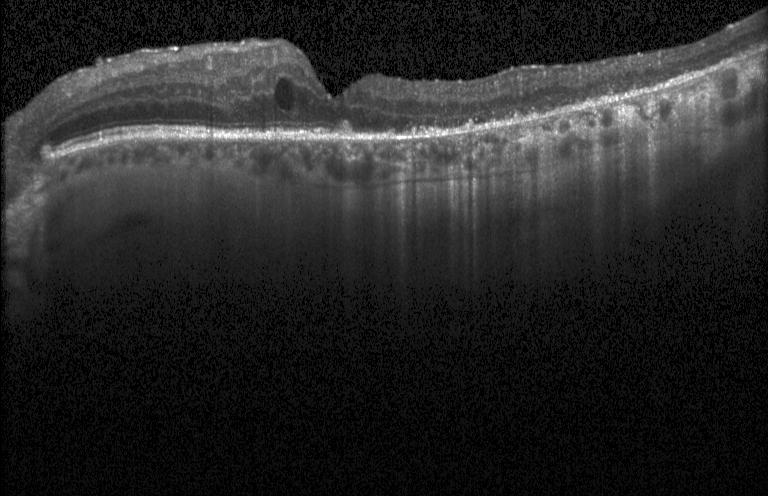
Instrument: Heidelberg Spectralis, OCT line scan, spectral-domain OCT, centered on the fovea.
OCT finding: diabetic macular edema (DME).